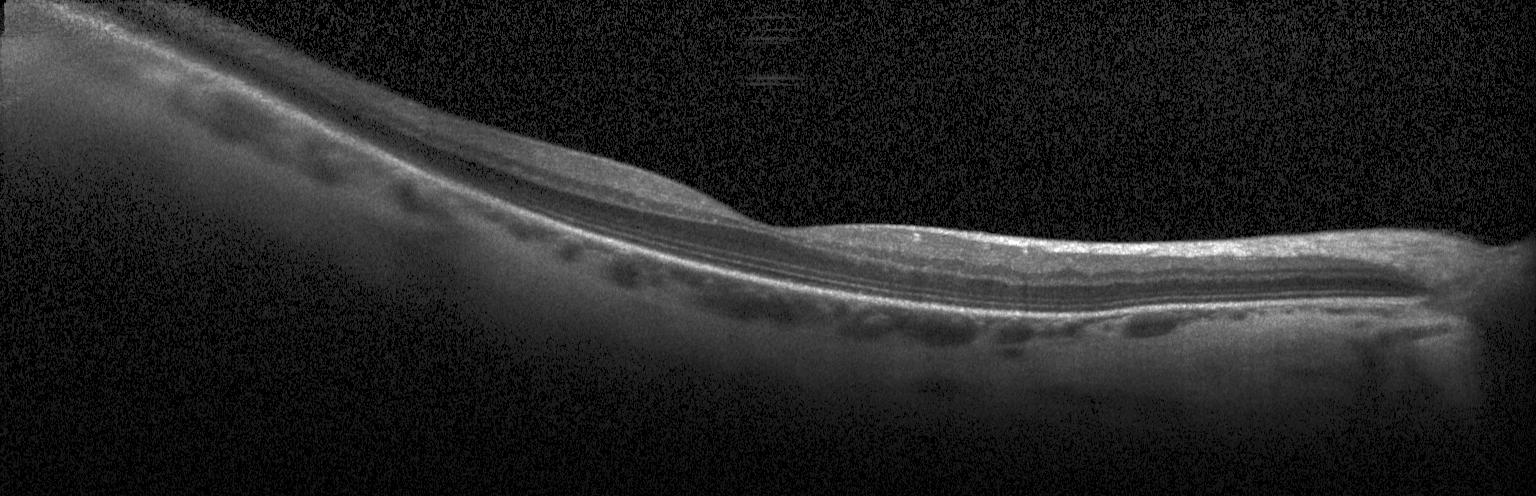 Instrument: Heidelberg Spectralis. Centered on the fovea. SD-OCT. Retinal OCT B-scan.
Impression: no choroidal neovascularization, no diabetic macular edema, and no drusen.